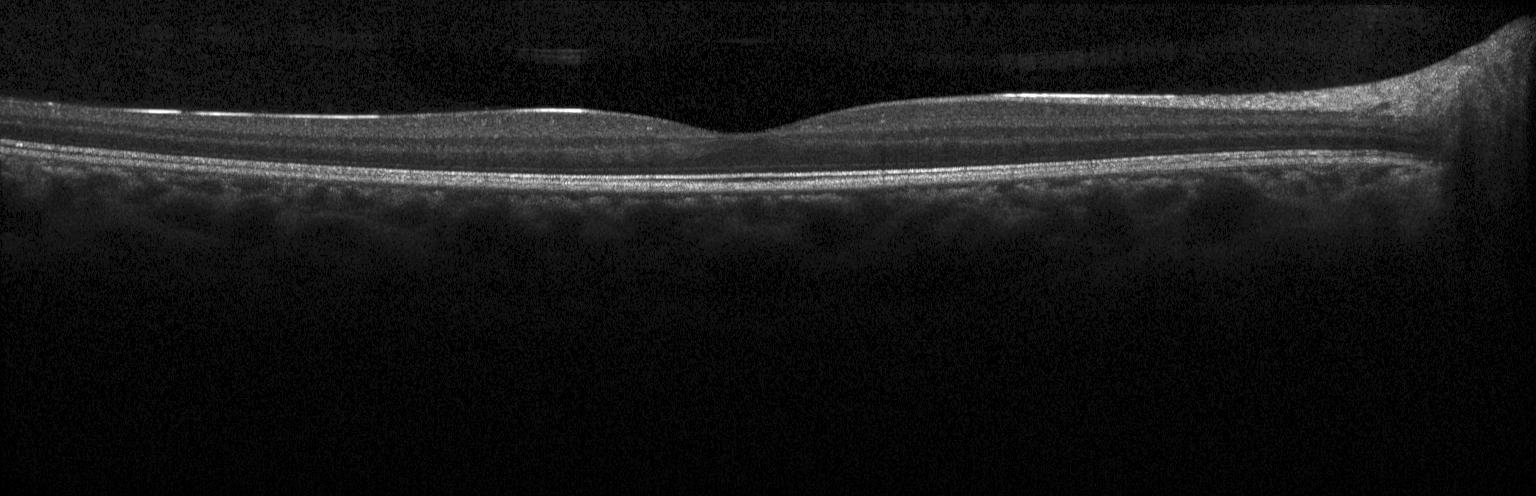
Macular scan; retinal OCT cross-section; instrument: Heidelberg Spectralis — This B-scan demonstrates no choroidal neovascularization, no diabetic macular edema, and no drusen.